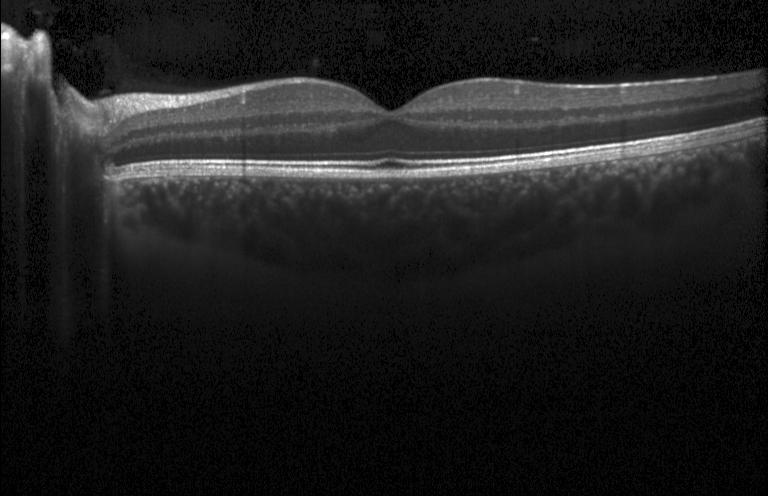

OCT B-scan. Impression: no CNV, DME, or drusen.